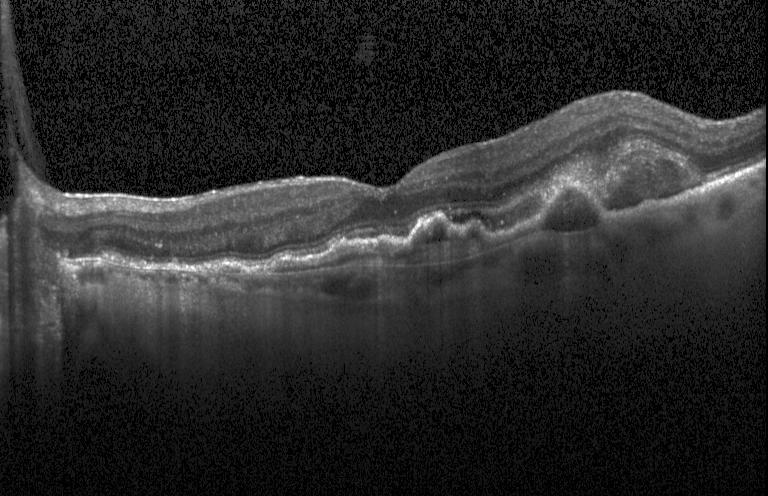 Impression: CNV.